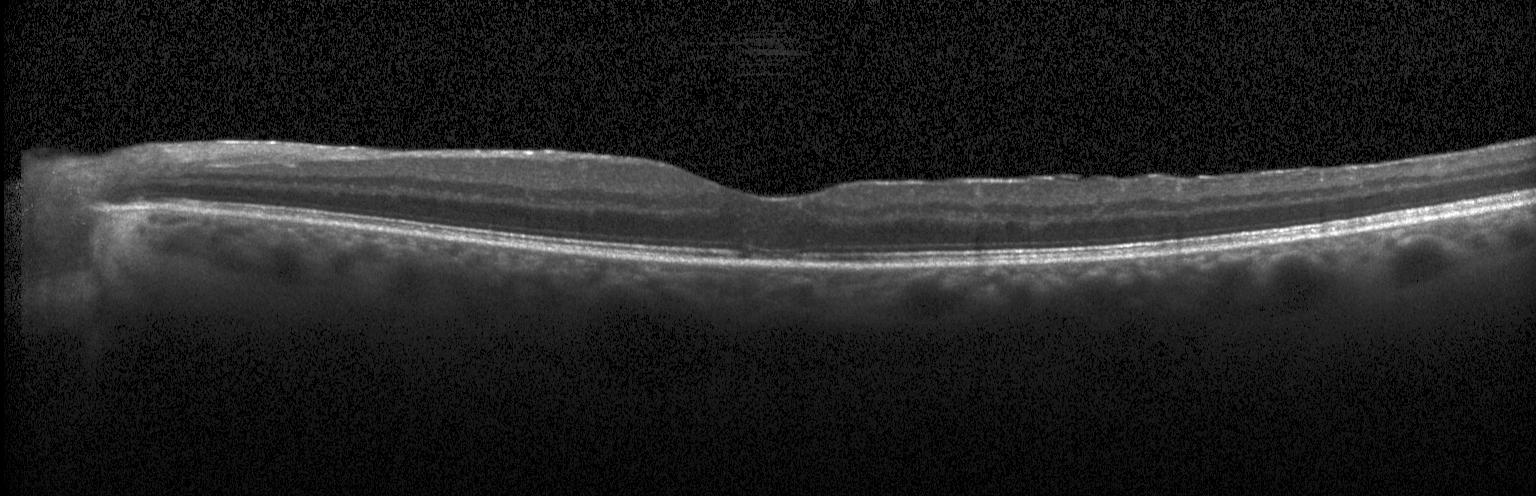 Diagnosis: no evidence of choroidal neovascularization, diabetic macular edema, or drusen.